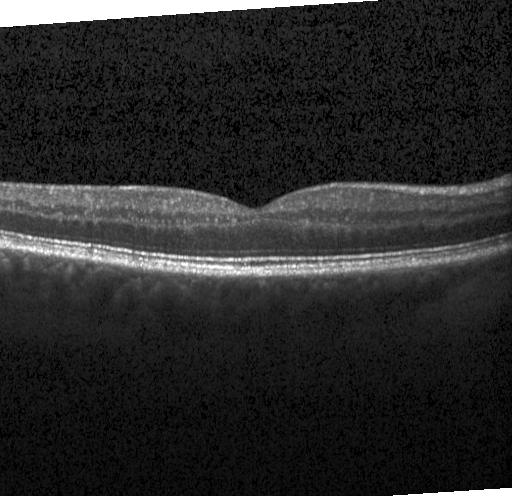 Optical coherence tomography B-scan.
Macular OCT: no CNV, DME, or drusen.